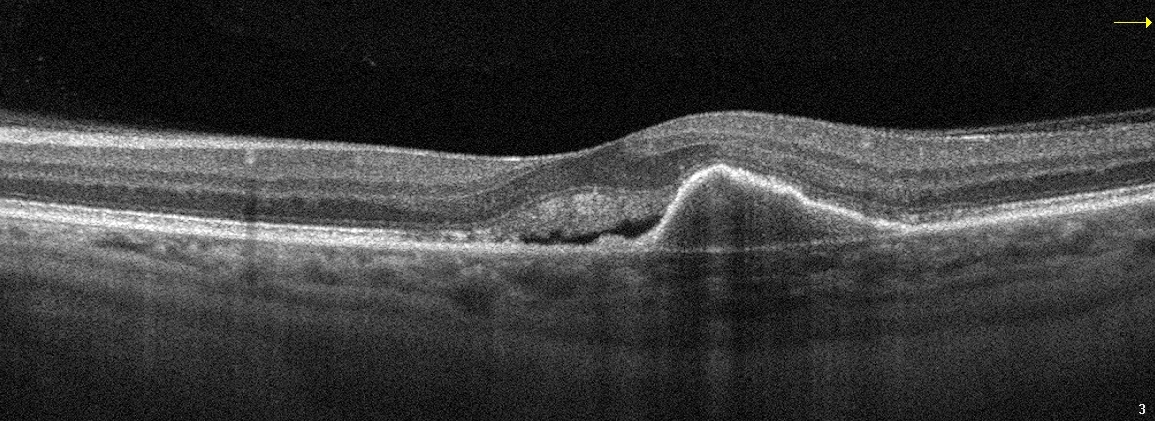 Retinal OCT B-scan — AMD.